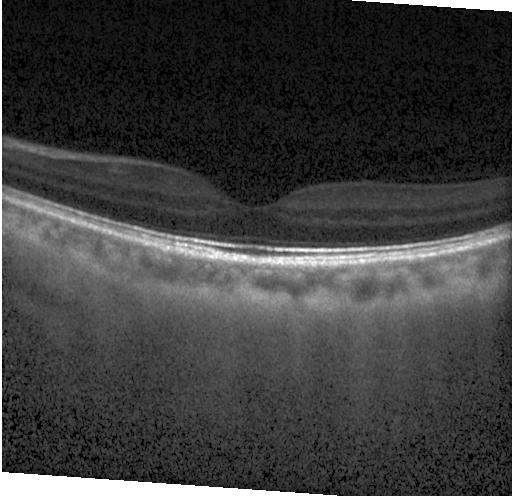
SD-OCT. Heidelberg Spectralis OCT system. OCT line scan. Horizontal scan through the fovea
The scan shows no choroidal neovascularization, no diabetic macular edema, and no drusen.